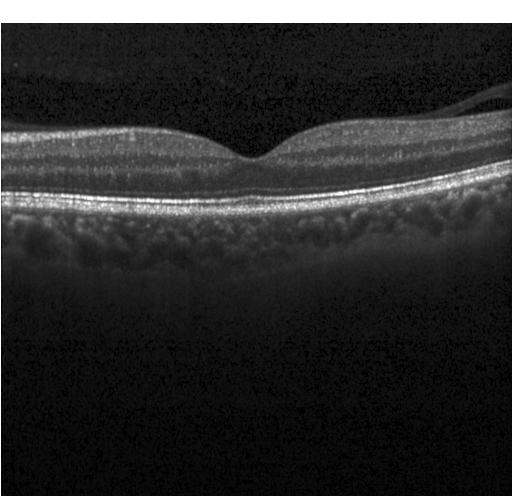 Macular OCT: neither choroidal neovascularization, diabetic macular edema, nor drusen.